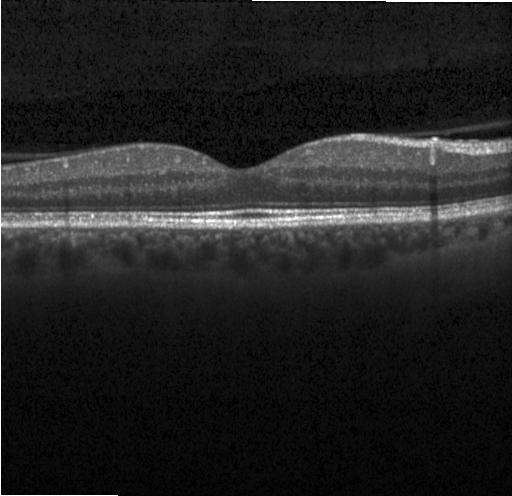
OCT line scan
Finding: no choroidal neovascularization, diabetic macular edema, or drusen.